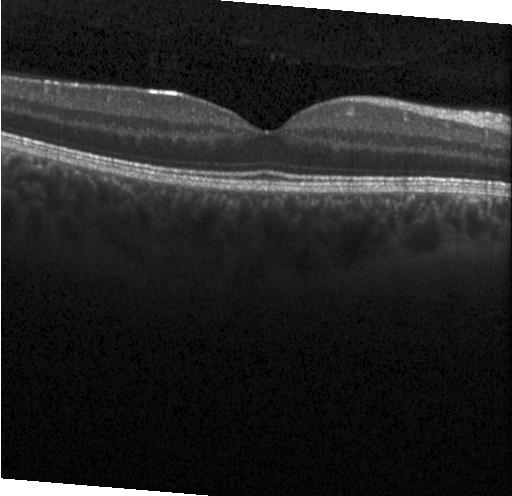 OCT scan showing no CNV, no DME, and no drusen.